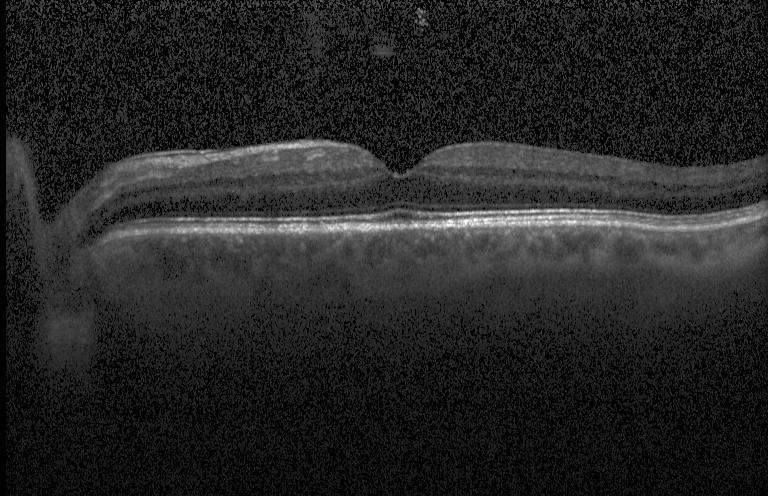

Heidelberg Spectralis. Horizontal scan through the fovea. Spectral-domain optical coherence tomography. Retinal OCT B-scan.
Dx: no evidence of choroidal neovascularization, diabetic macular edema, or drusen.